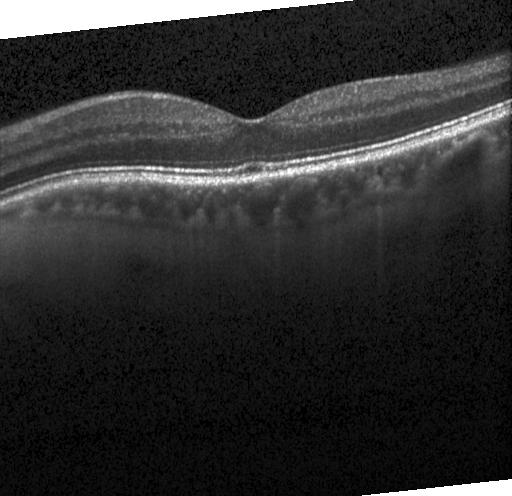
Impression: no choroidal neovascularization, no diabetic macular edema, and no drusen.